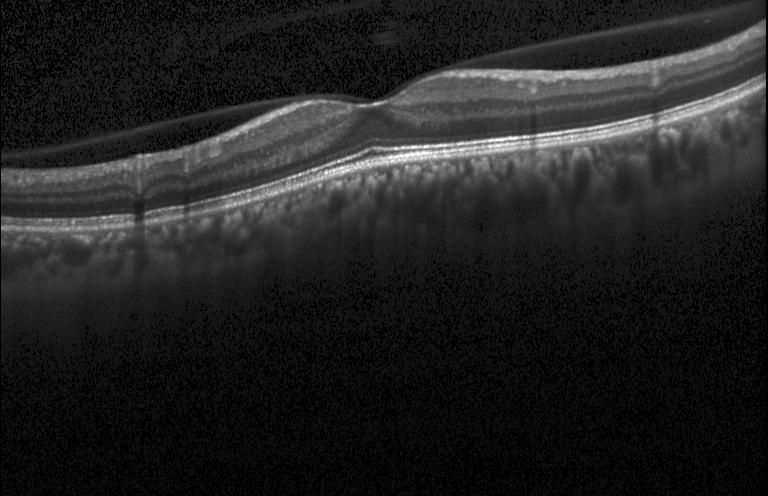 Optical coherence tomography scan; instrument: Heidelberg Spectralis
This B-scan demonstrates no CNV, no DME, and no drusen.